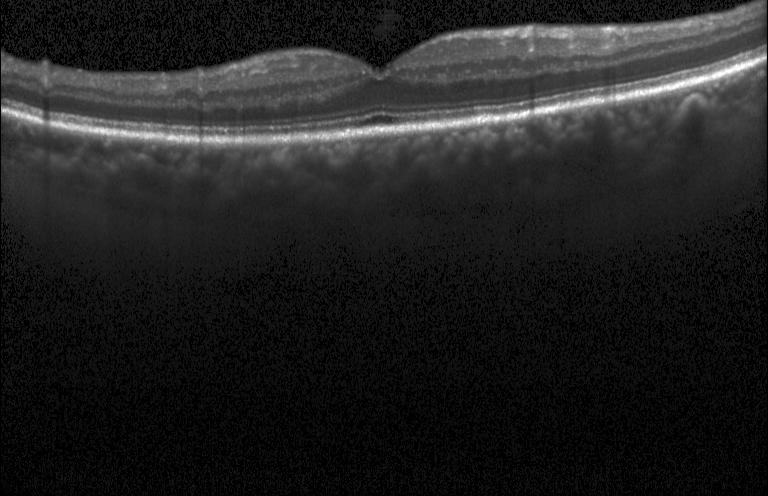
No choroidal neovascularization, diabetic macular edema, or drusen.